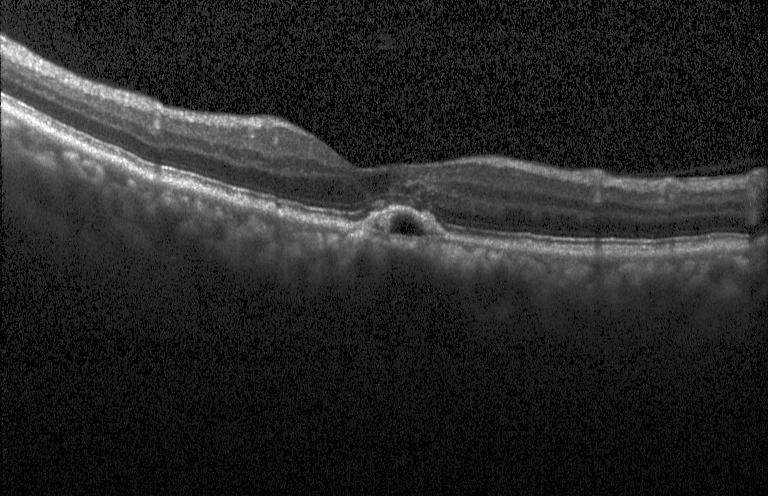

Retinal OCT cross-section
The scan shows a choroidal neovascular membrane.